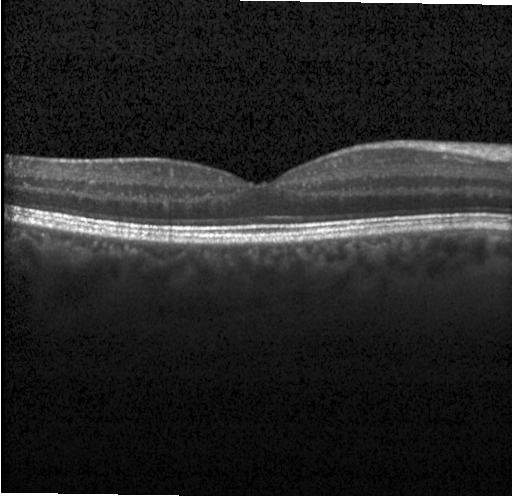

Heidelberg Spectralis; OCT B-scan. Diagnosis: no choroidal neovascularization, diabetic macular edema, or drusen.